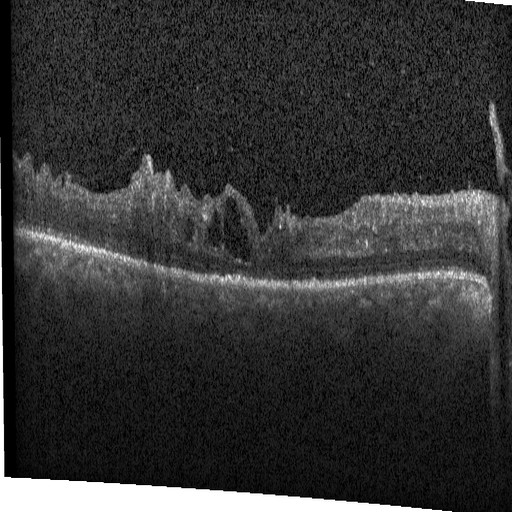

OCT B-scan showing diabetic macular edema.